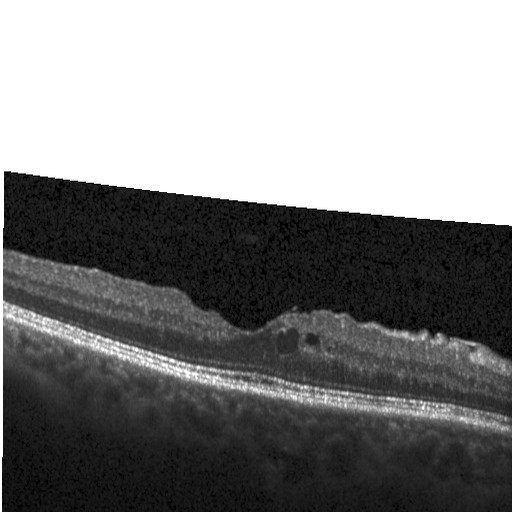

Spectral-domain OCT B-scan: diabetic macular edema.